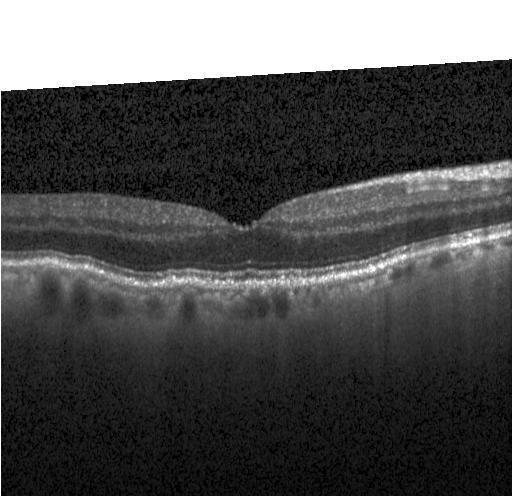 Retinal OCT B-scan · Heidelberg Spectralis OCT system · centered on the fovea · spectral-domain OCT
OCT finding: sub-RPE drusenoid deposits.